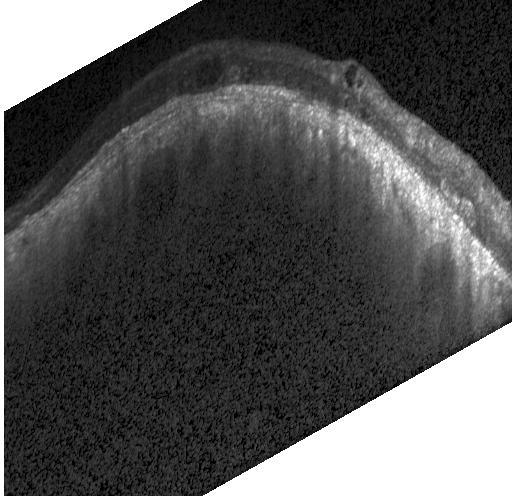
OCT line scan. Horizontal scan through the fovea
Assessment: DME.